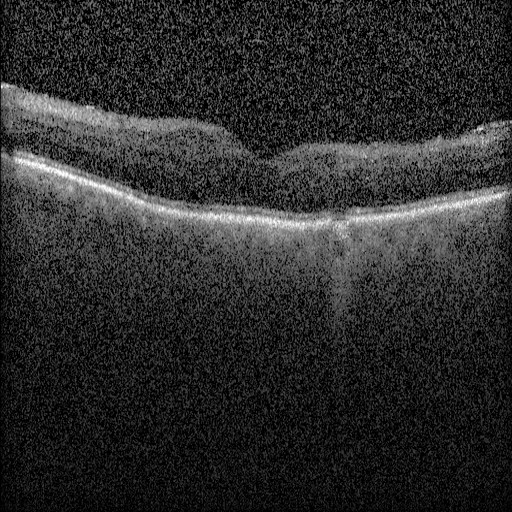 Finding: DME.